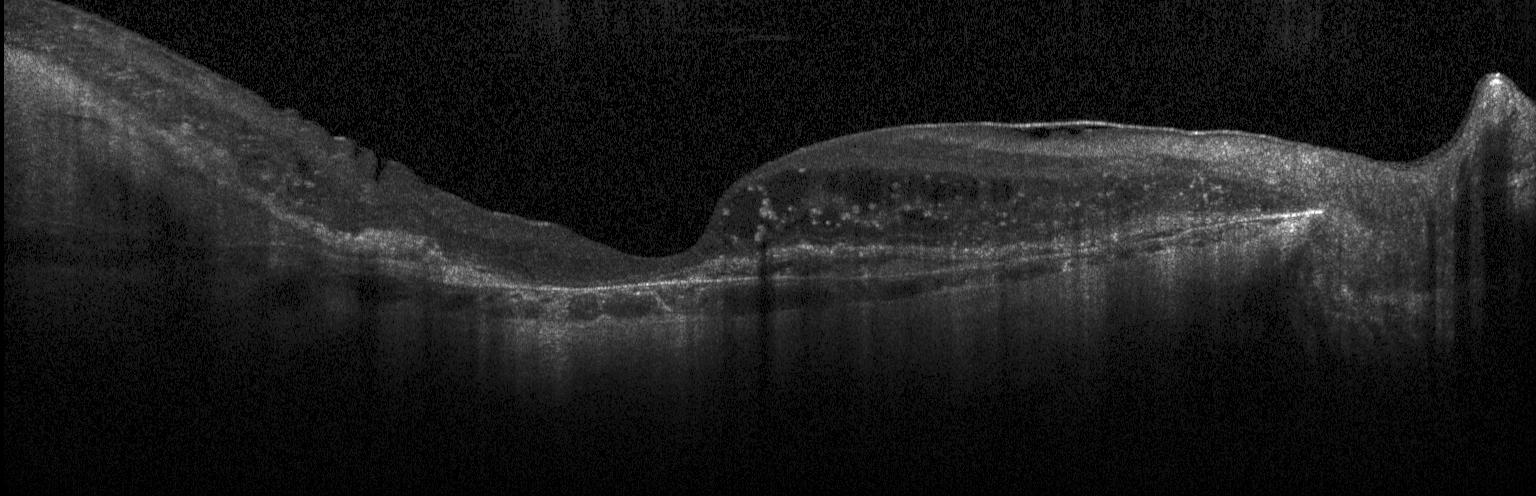

Optical coherence tomography B-scan.
Assessment: a choroidal neovascular membrane.